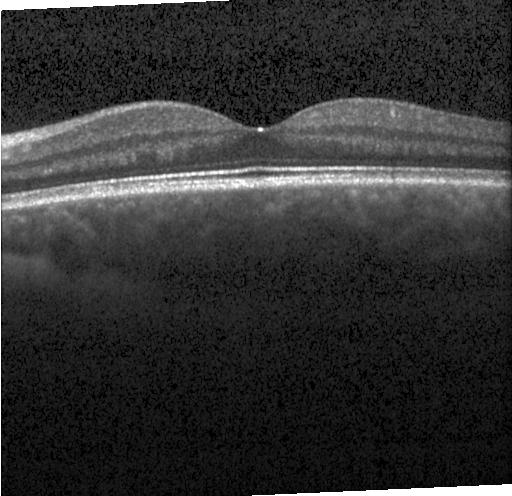
Finding: no choroidal neovascularization, diabetic macular edema, or drusen.